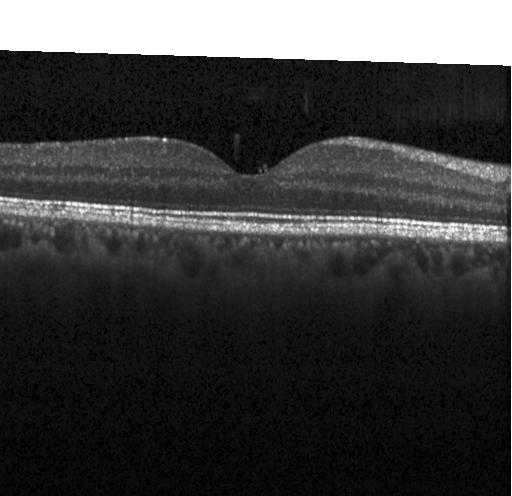

Instrument: Heidelberg Spectralis. Retinal OCT cross-section. Fovea-centered
Dx: neither CNV, DME, nor drusen.